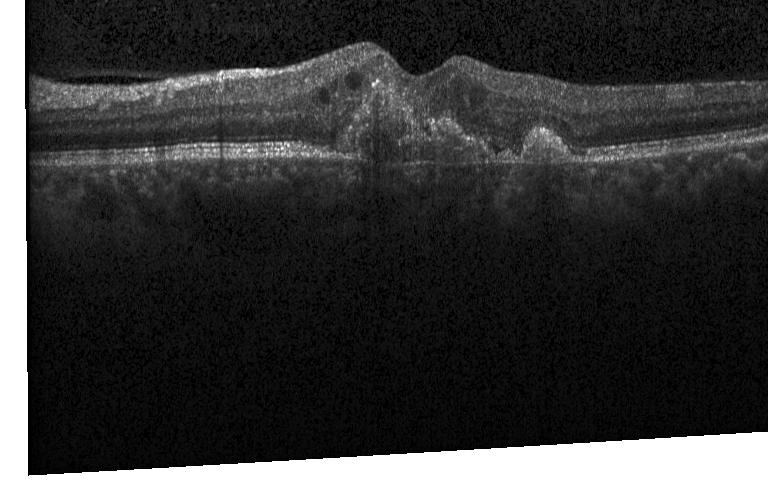

Optical coherence tomography scan; SD-OCT
Diagnosis: CNV.